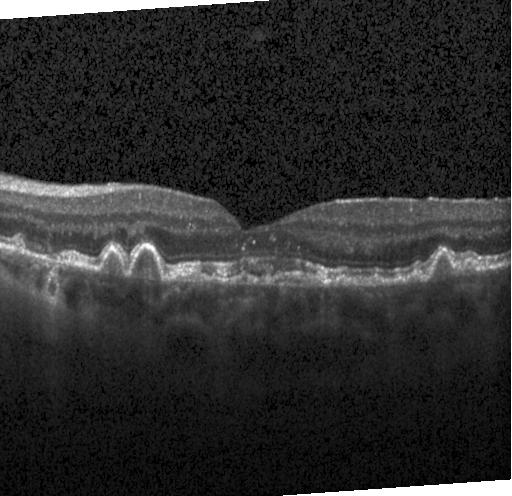

Acquired on a Heidelberg Spectralis · spectral-domain optical coherence tomography · optical coherence tomography scan. Finding: a choroidal neovascular membrane.